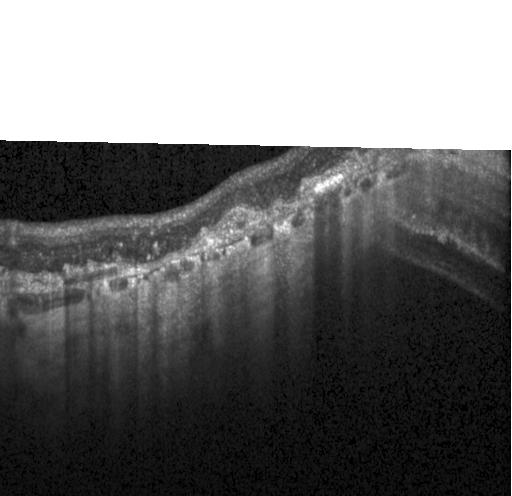
Macular scan, Heidelberg Spectralis, SD-OCT, OCT line scan. A choroidal neovascular membrane.